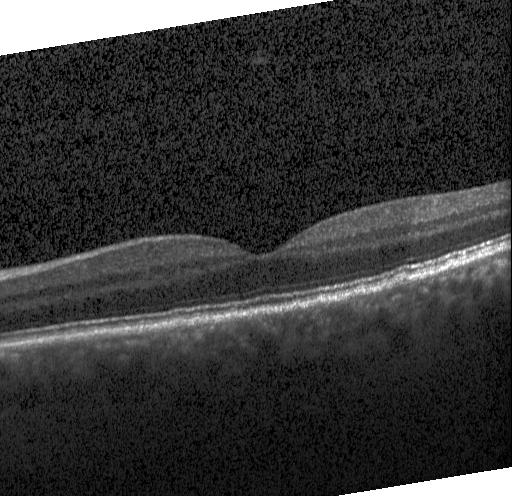 Spectral-domain OCT. OCT line scan. Fovea-centered — Macular OCT: multiple drusen.